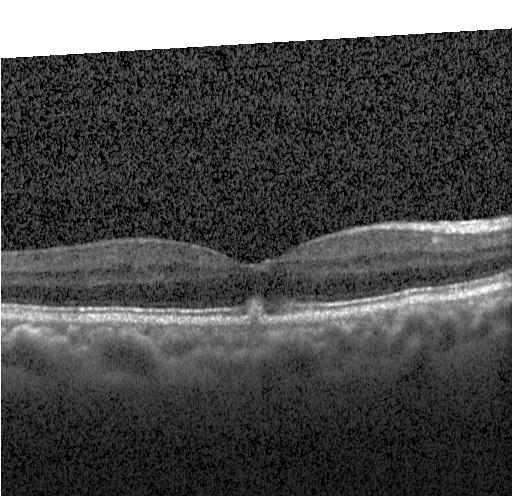
Diagnosis: sub-RPE drusenoid deposits.